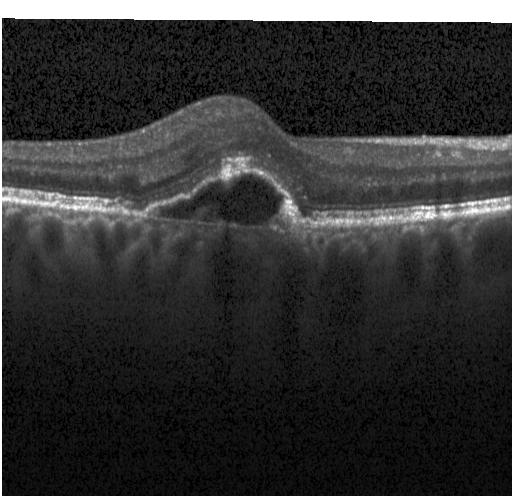 SD-OCT, Heidelberg Spectralis OCT system, centered on the fovea, optical coherence tomography scan — Finding: choroidal neovascularization (CNV).